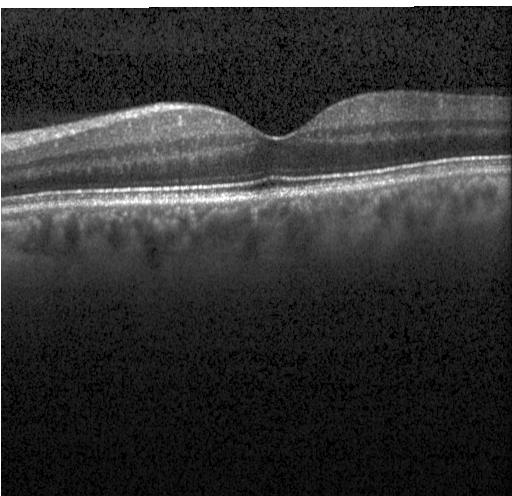
Diagnosis: no evidence of CNV, DME, or drusen.